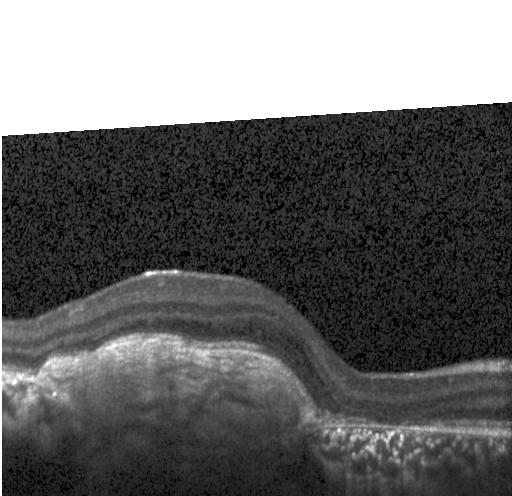
Spectral-domain OCT, OCT B-scan, fovea-centered, Heidelberg Spectralis.
Finding: choroidal neovascularization.